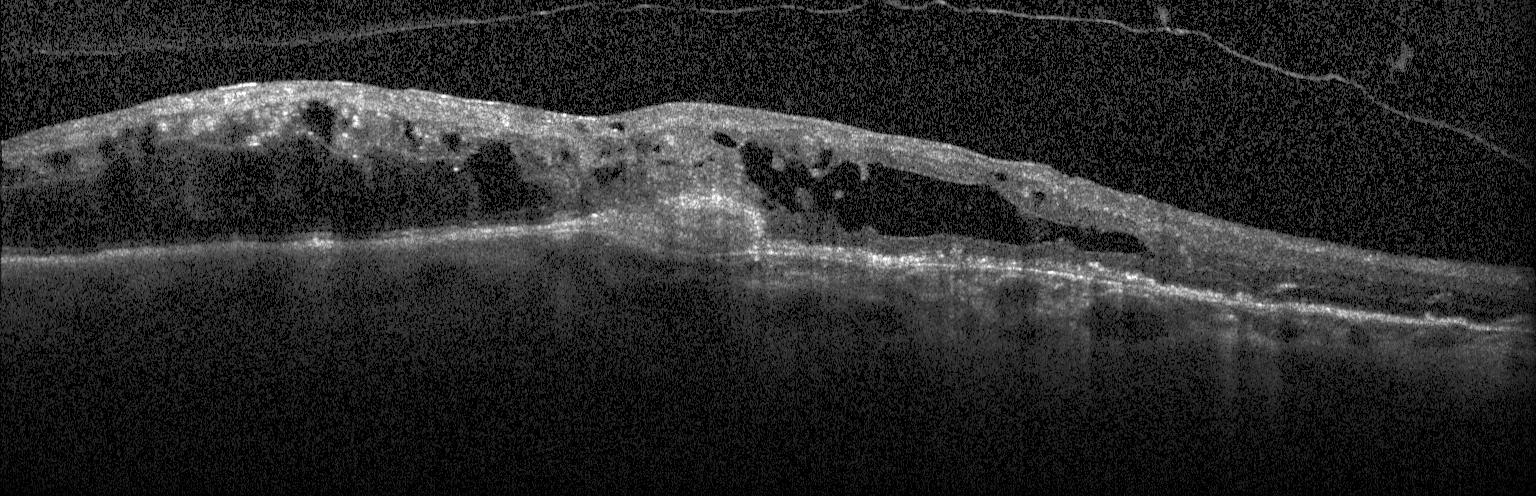
Macular OCT: choroidal neovascularization (CNV).